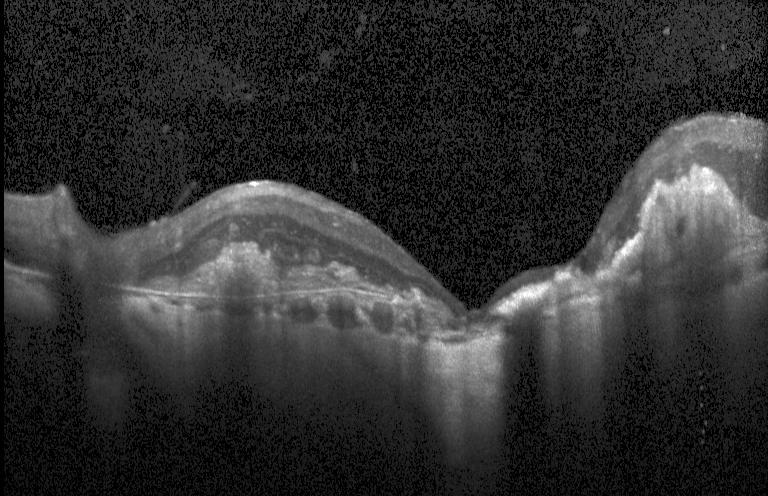
OCT finding: a choroidal neovascular membrane.